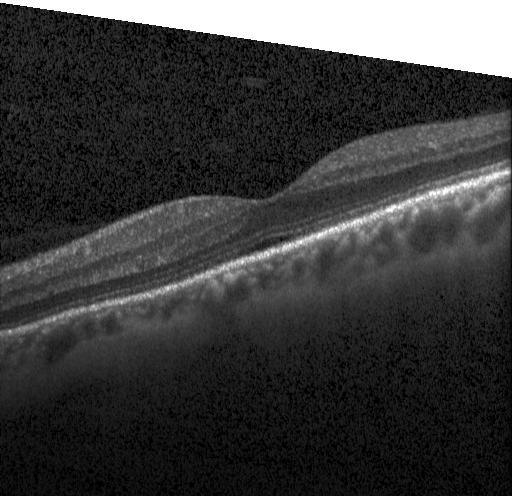
Optical coherence tomography B-scan, fovea-centered.
Neither choroidal neovascularization, diabetic macular edema, nor drusen.